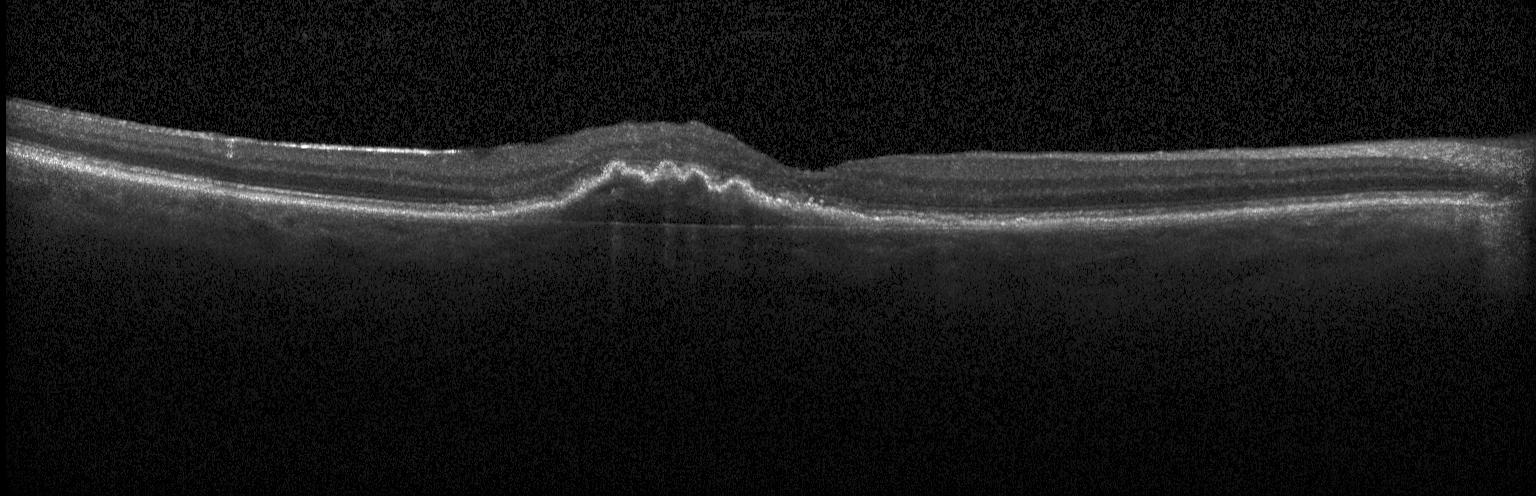

Fovea-centered. OCT B-scan. Heidelberg Spectralis. Spectral-domain OCT — Macular OCT: choroidal neovascularization (CNV).